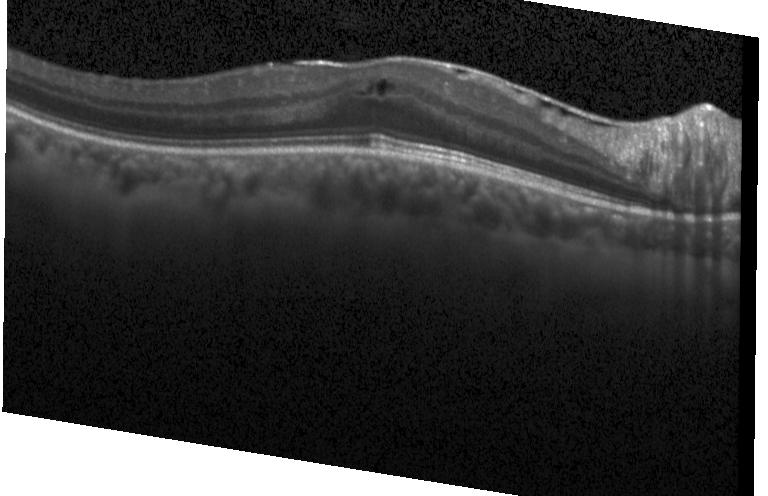
Through the macula. OCT B-scan
Assessment: DME.